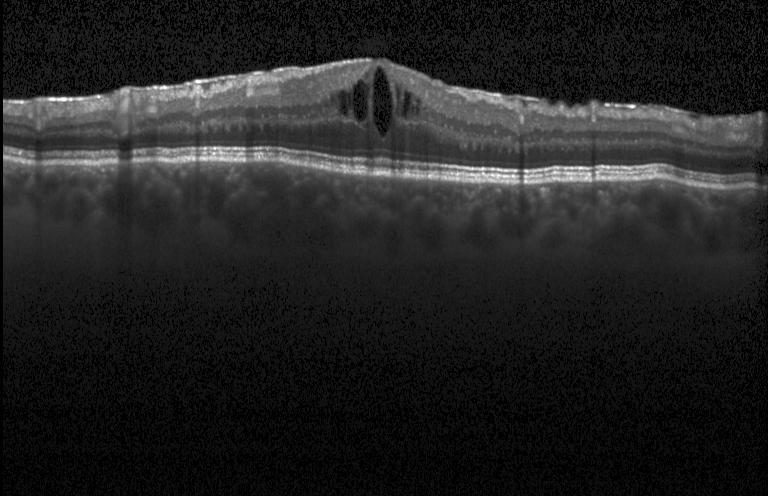 Macular OCT: DME.